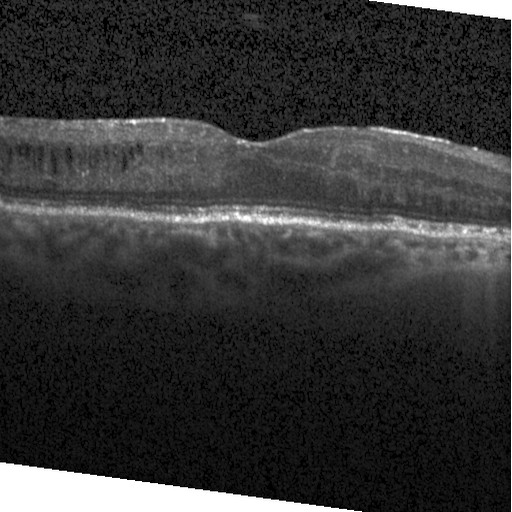
Spectral-domain OCT B-scan: diabetic macular edema.